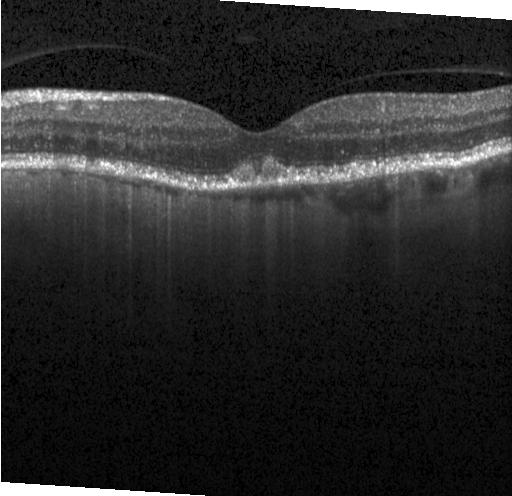 Retinal OCT cross-section
Sub-RPE drusenoid deposits.